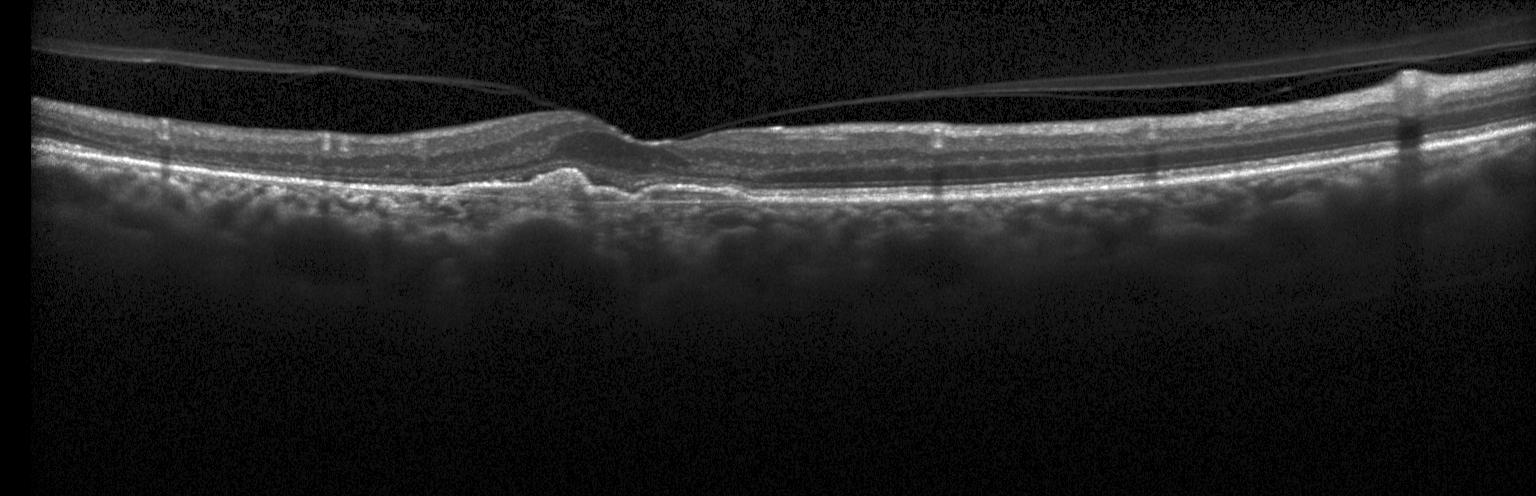

The scan shows a choroidal neovascular membrane.